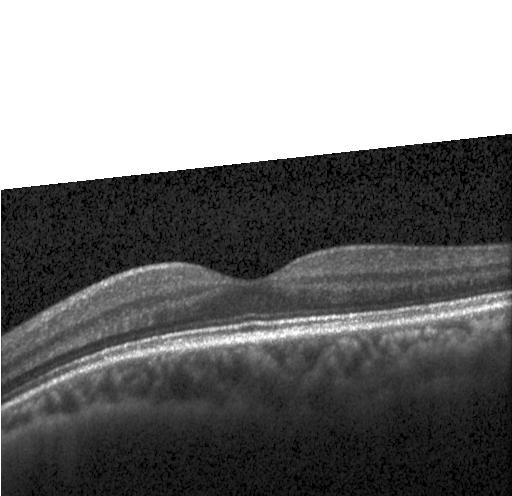
OCT finding: no evidence of choroidal neovascularization, diabetic macular edema, or drusen.